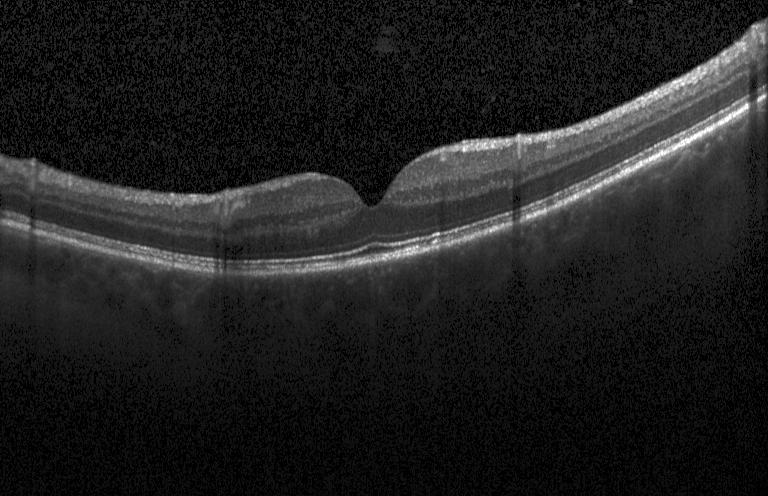

Spectral-domain OCT, Heidelberg Spectralis OCT system, retinal OCT cross-section — The scan shows no evidence of CNV, DME, or drusen.